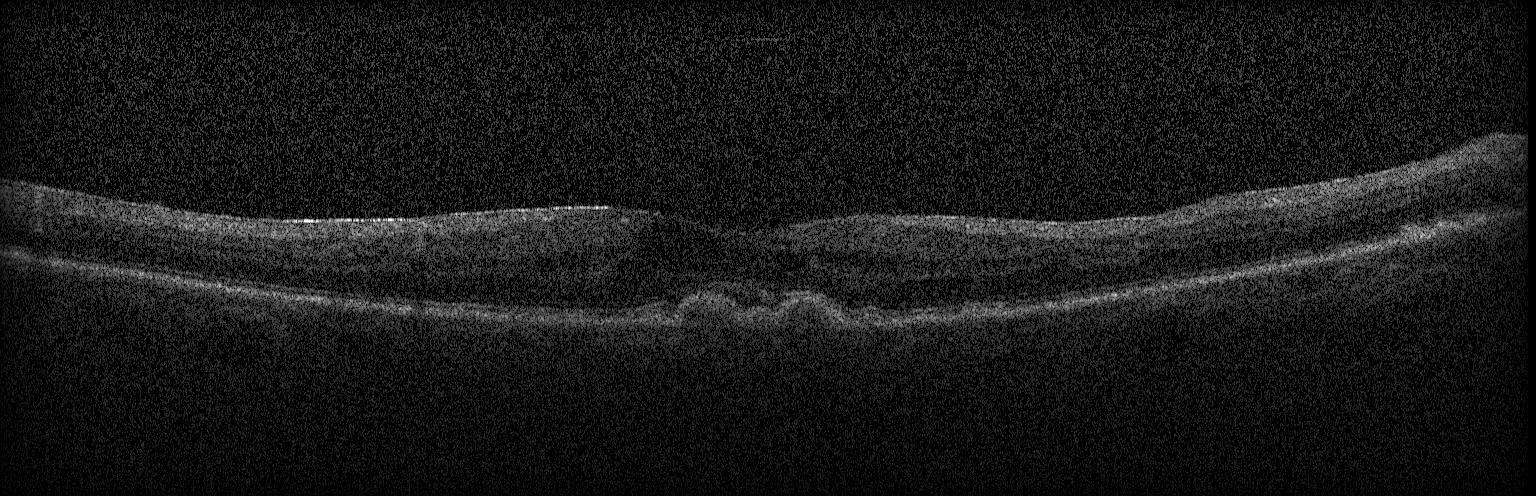

OCT line scan.
OCT finding: a choroidal neovascular membrane.